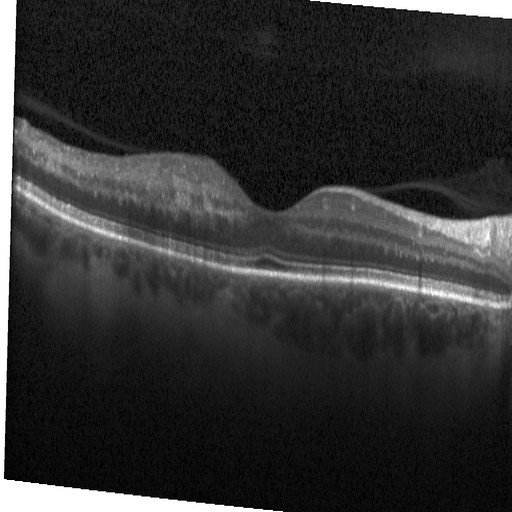
Macular scan. Optical coherence tomography scan. Spectral-domain OCT — DME.